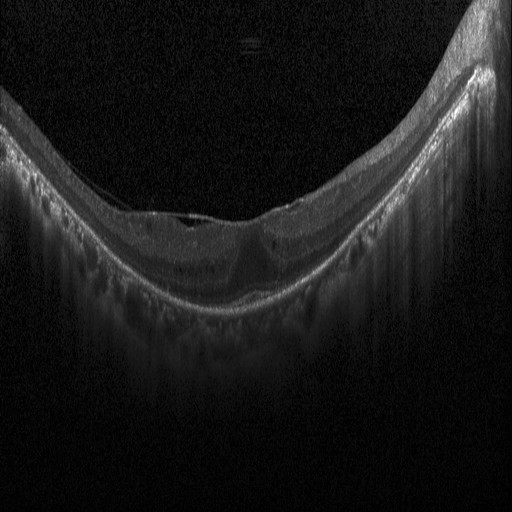 Macular scan. Heidelberg Spectralis OCT system. Retinal OCT B-scan. Dx: diabetic macular edema.